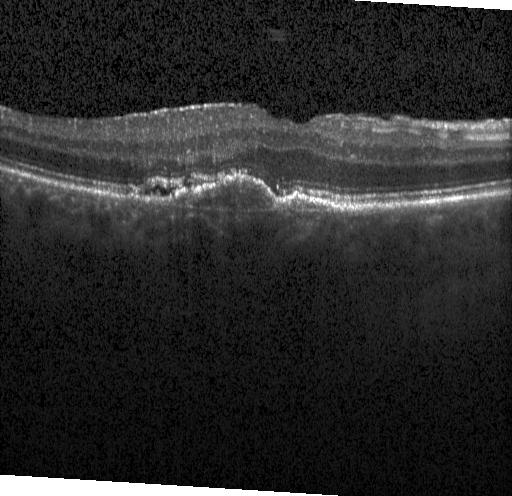
Centered on the fovea · Heidelberg Spectralis OCT system · OCT line scan · spectral-domain optical coherence tomography
Diagnosis: a choroidal neovascular membrane.